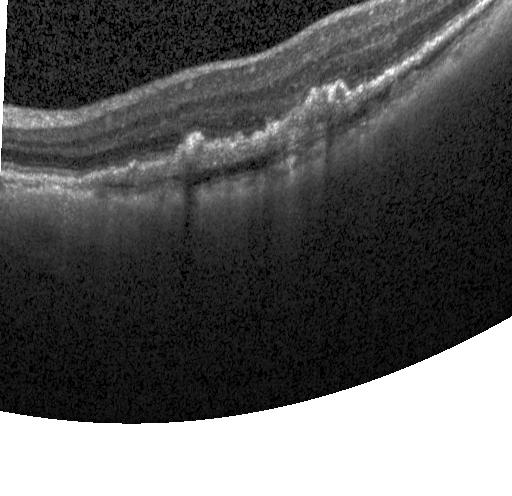 OCT B-scan · macular scan · Heidelberg Spectralis
Diagnosis: choroidal neovascularization (CNV).